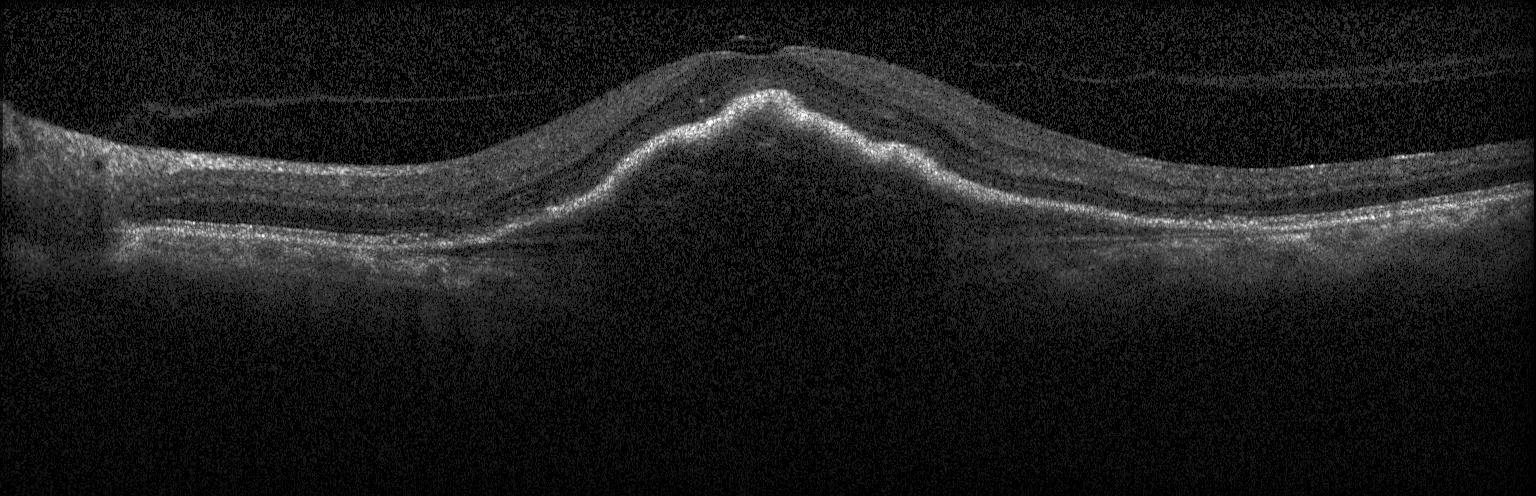

OCT B-scan showing CNV.